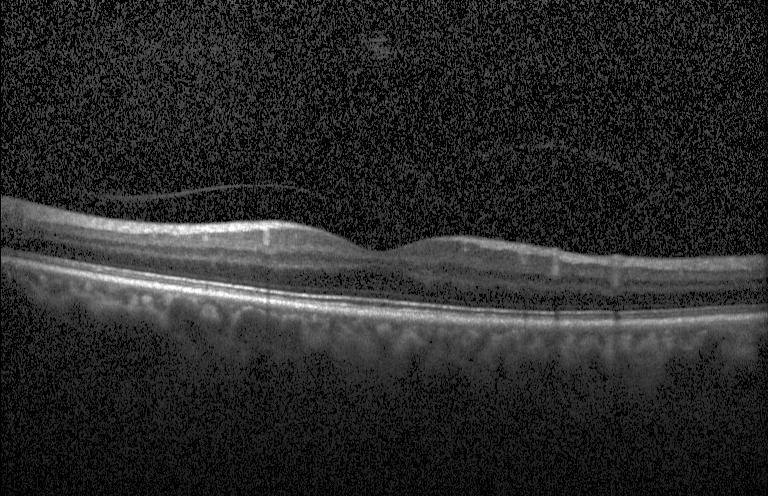

Optical coherence tomography B-scan, centered on the fovea, Heidelberg Spectralis, spectral-domain optical coherence tomography
Impression: neither CNV, DME, nor drusen.